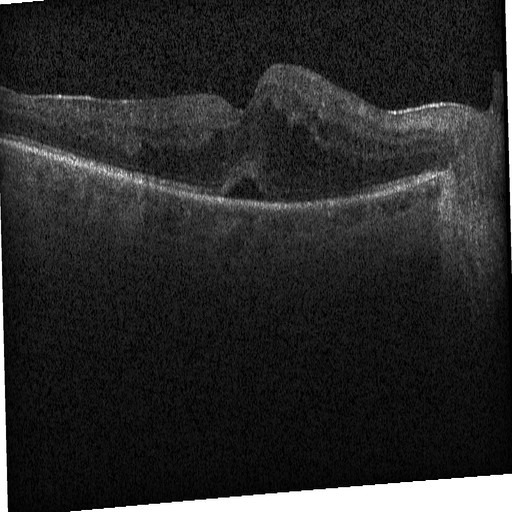 Finding: diabetic macular edema.